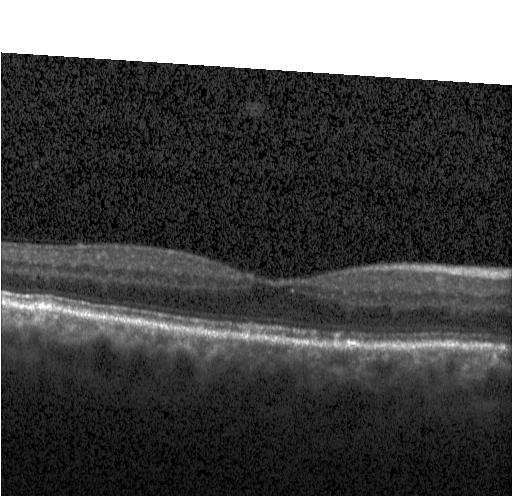

Centered on the fovea, acquired on a Heidelberg Spectralis, SD-OCT, OCT B-scan — Diagnosis: no evidence of choroidal neovascularization, diabetic macular edema, or drusen.